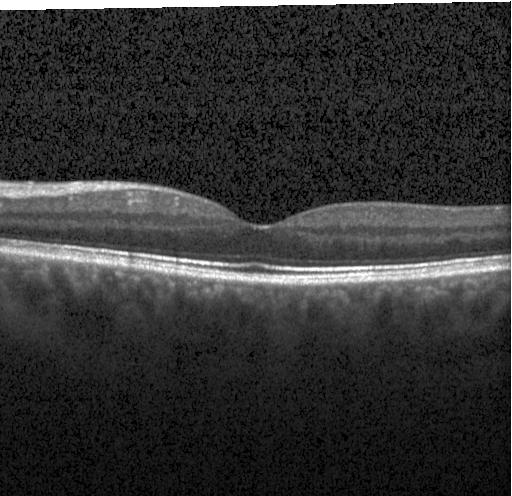
Retinal OCT cross-section showing no choroidal neovascularization, diabetic macular edema, or drusen.